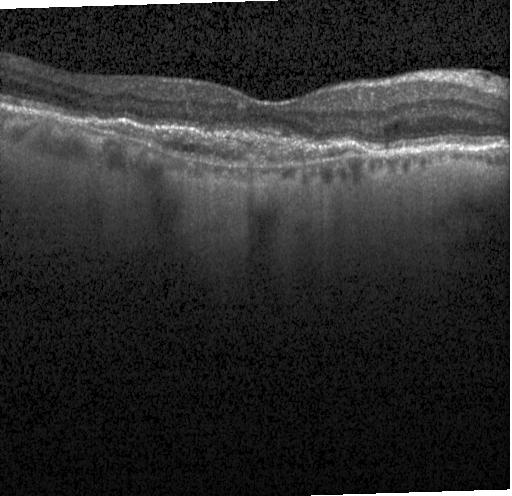 Spectral-domain OCT B-scan: choroidal neovascularization.